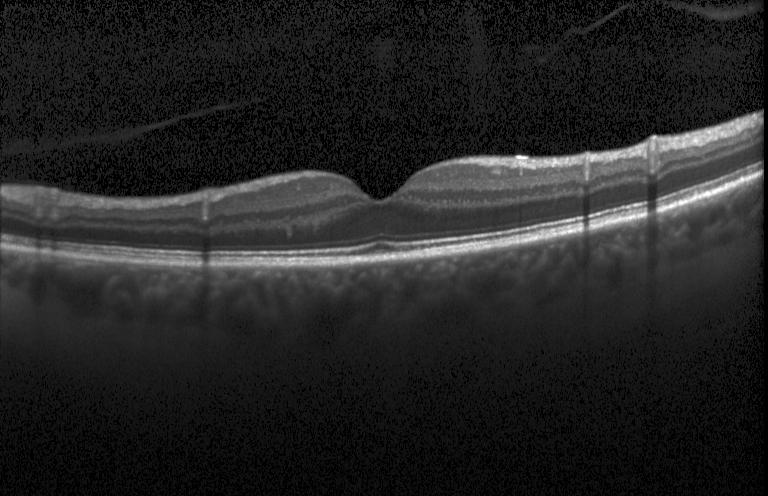 Fovea-centered; OCT B-scan — Dx: neither choroidal neovascularization, diabetic macular edema, nor drusen.